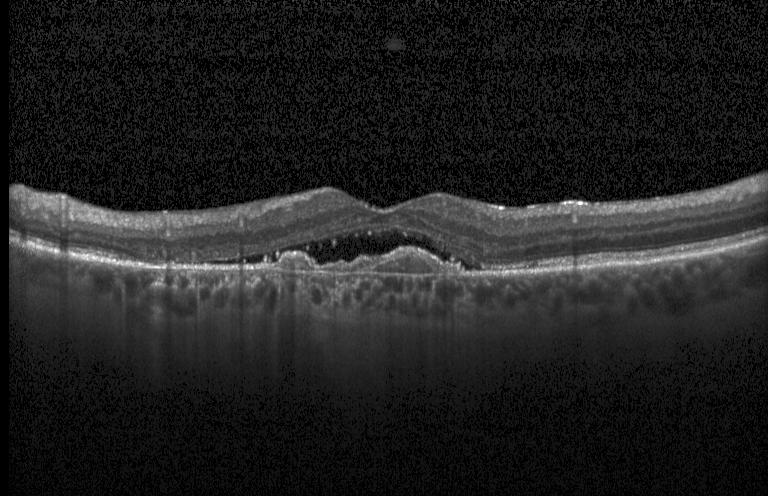
Retinal OCT cross-section · Heidelberg Spectralis OCT system · macular scan · spectral-domain OCT
Impression: a choroidal neovascular membrane.